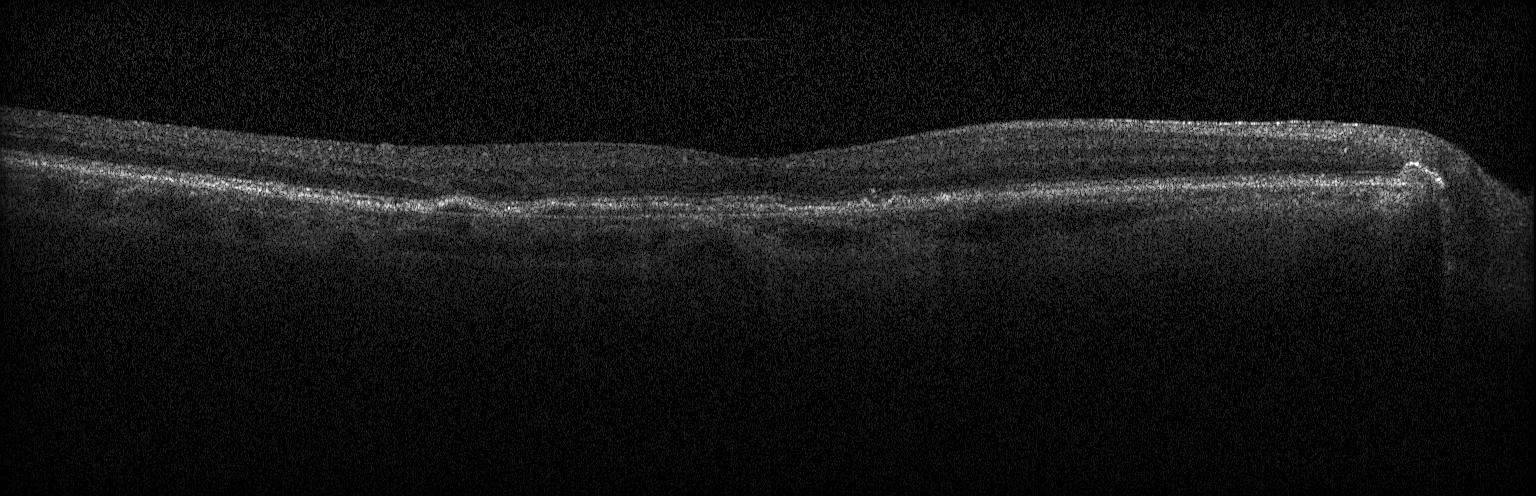
Finding: a choroidal neovascular membrane.